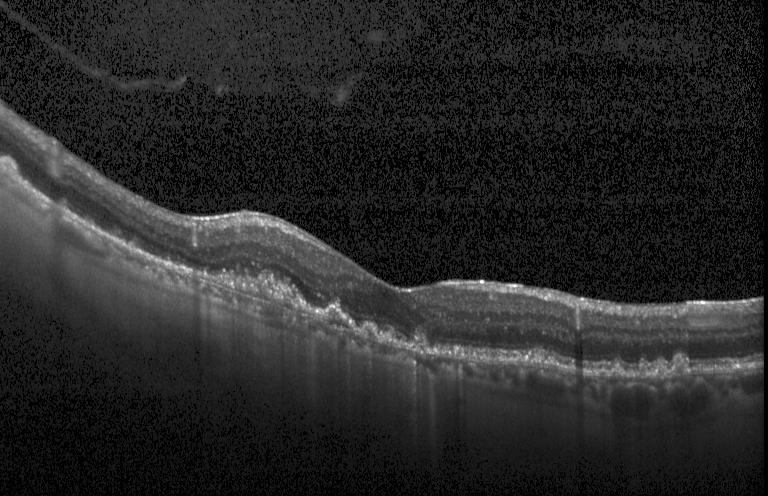 Optical coherence tomography scan · instrument: Heidelberg Spectralis · through the macula.
Finding: choroidal neovascularization (CNV).